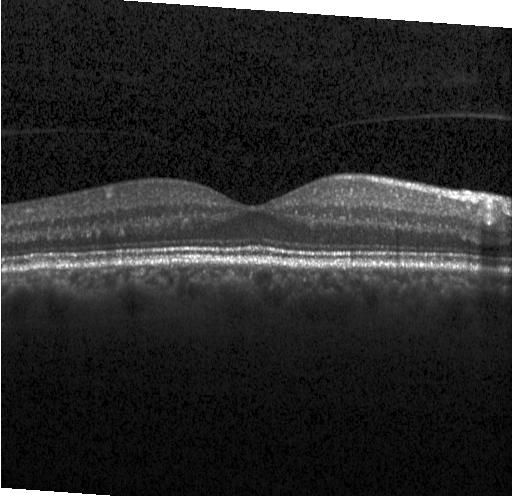
Horizontal scan through the fovea, optical coherence tomography B-scan, spectral-domain optical coherence tomography.
Finding: neither choroidal neovascularization, diabetic macular edema, nor drusen.